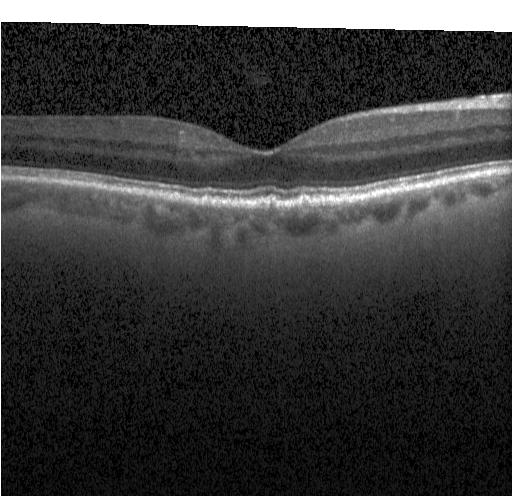
Optical coherence tomography scan.
Assessment: sub-RPE drusenoid deposits.